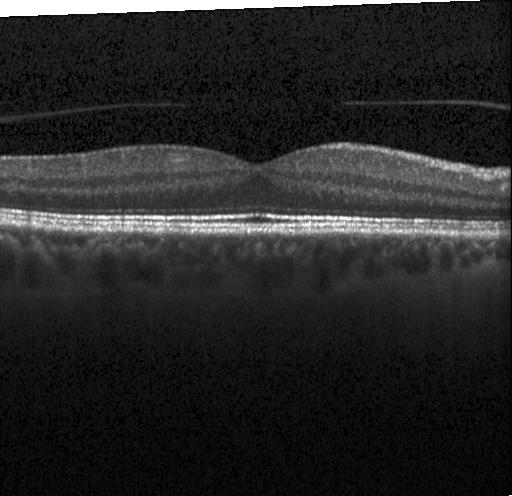
Spectral-domain OCT · retinal OCT cross-section. Impression: no CNV, DME, or drusen.